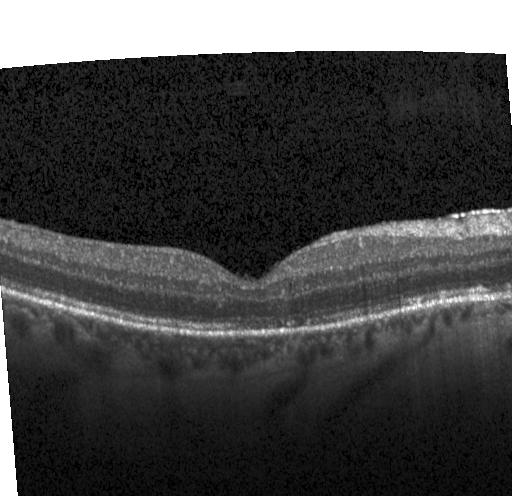 Finding: neither choroidal neovascularization, diabetic macular edema, nor drusen.